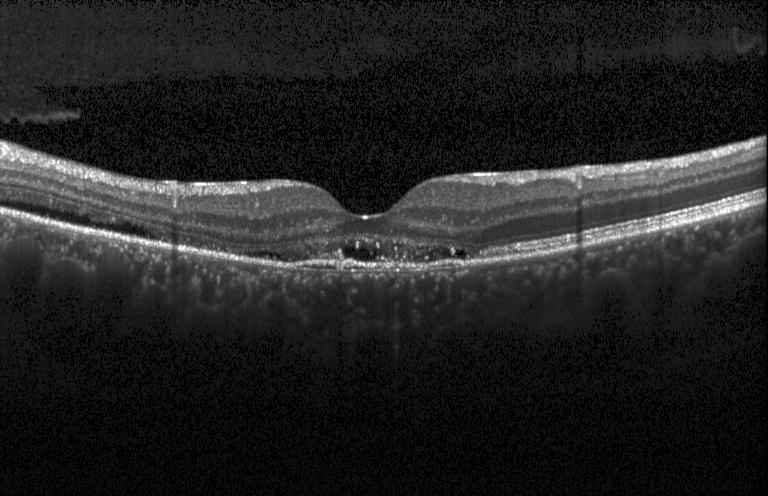
OCT line scan. Diagnosis: choroidal neovascularization.